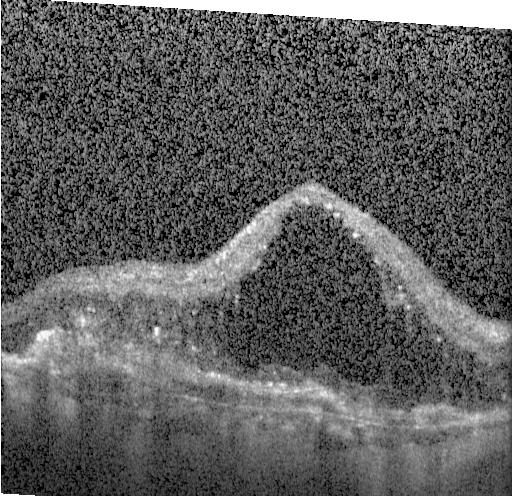

Spectral-domain OCT B-scan: a choroidal neovascular membrane.